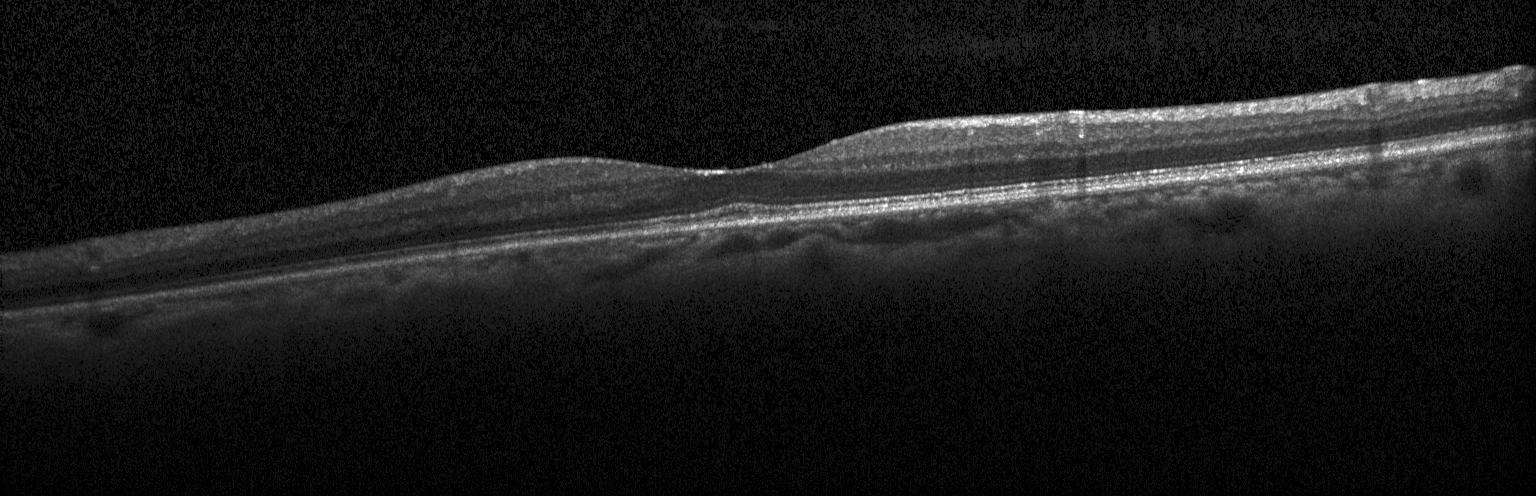

Retinal OCT cross-section
Diagnosis: no CNV, no DME, and no drusen.